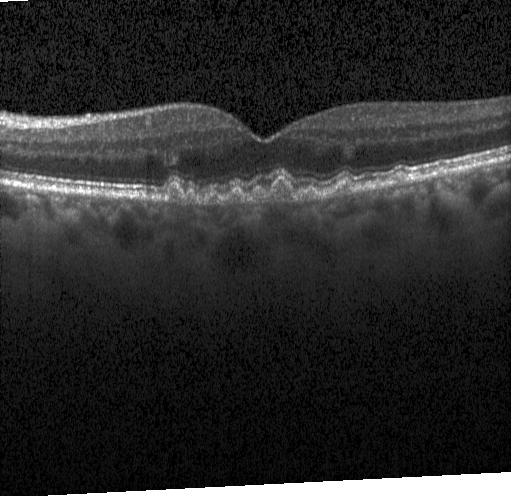 Acquired on a Heidelberg Spectralis; OCT B-scan; horizontal scan through the fovea. Diagnosis: multiple drusen.